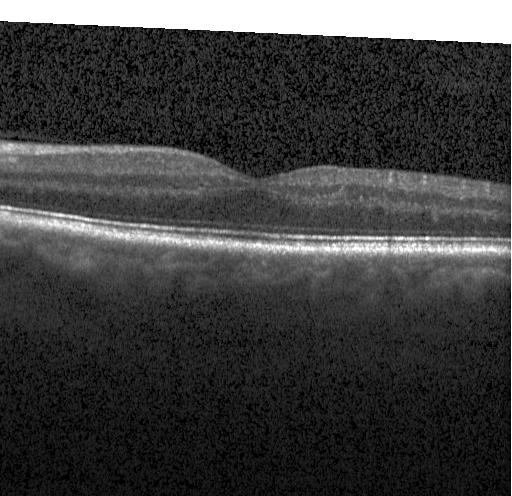

The scan shows no choroidal neovascularization, no diabetic macular edema, and no drusen.